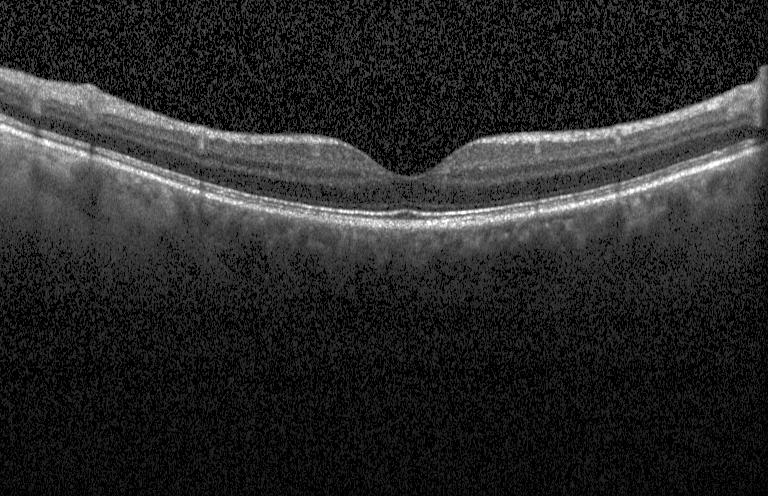 Finding: neither CNV, DME, nor drusen.